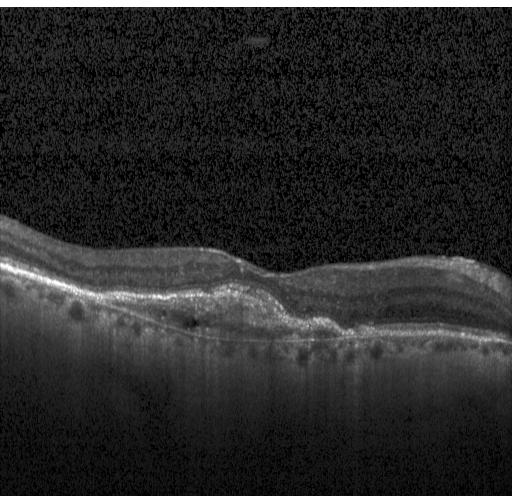

Optical coherence tomography scan; spectral-domain OCT. Finding: choroidal neovascularization (CNV).